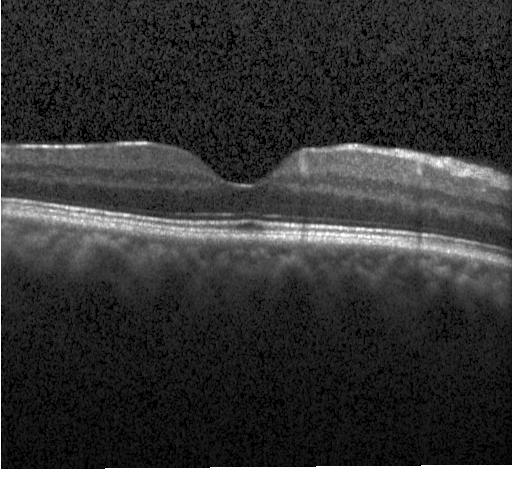 OCT finding: no evidence of choroidal neovascularization, diabetic macular edema, or drusen.